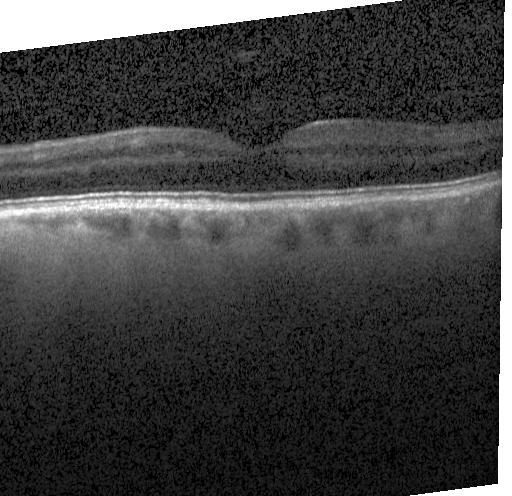

Dx: neither CNV, DME, nor drusen.